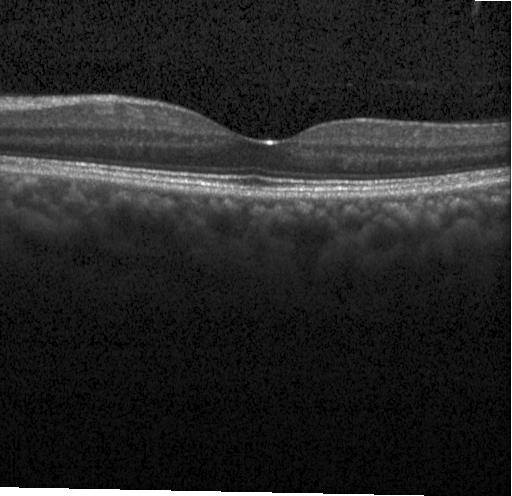
Diagnosis: neither choroidal neovascularization, diabetic macular edema, nor drusen.